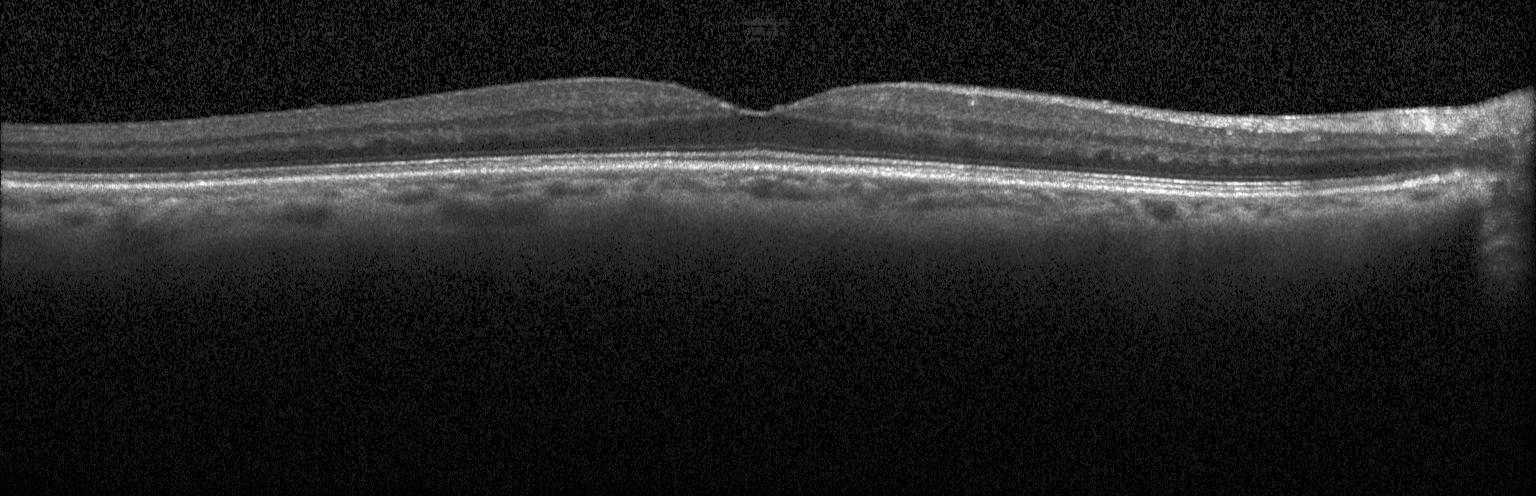

No evidence of choroidal neovascularization, diabetic macular edema, or drusen.